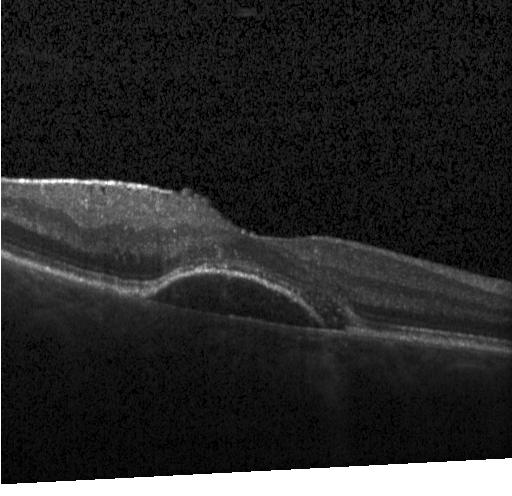

This B-scan demonstrates a choroidal neovascular membrane.